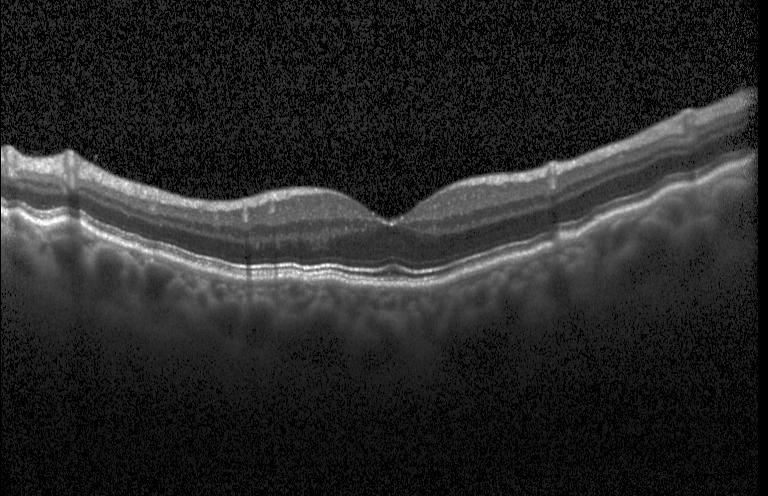

Optical coherence tomography scan. Heidelberg Spectralis OCT system
Assessment: no evidence of choroidal neovascularization, diabetic macular edema, or drusen.